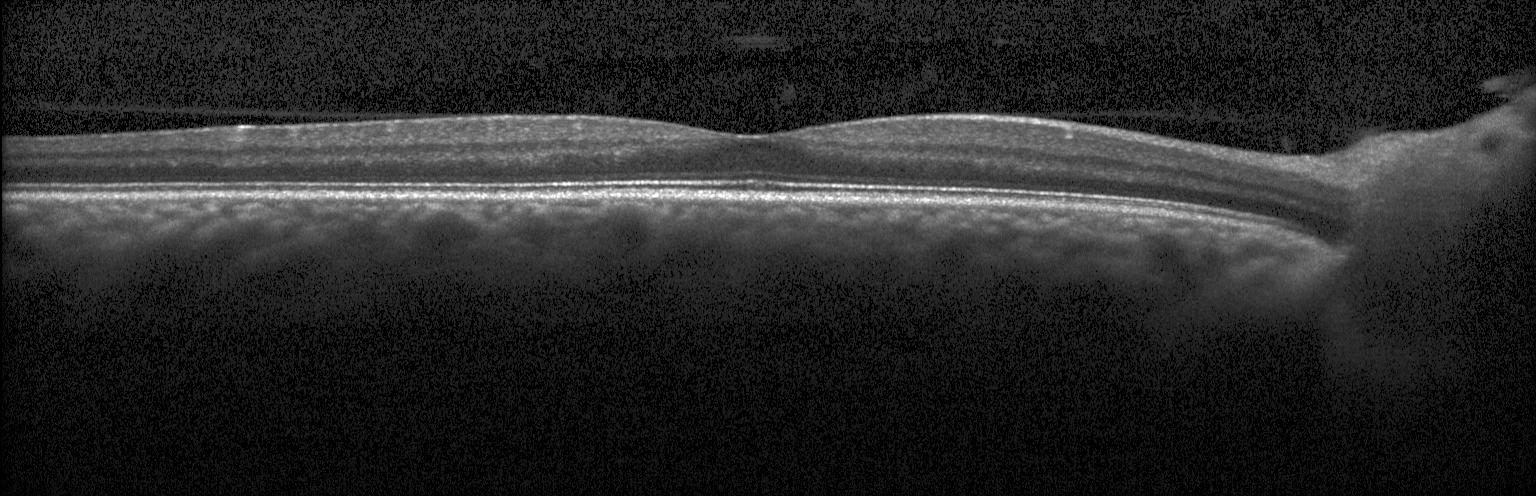 Spectral-domain OCT, OCT B-scan, acquired on a Heidelberg Spectralis, through the macula. OCT finding: no choroidal neovascularization, no diabetic macular edema, and no drusen.